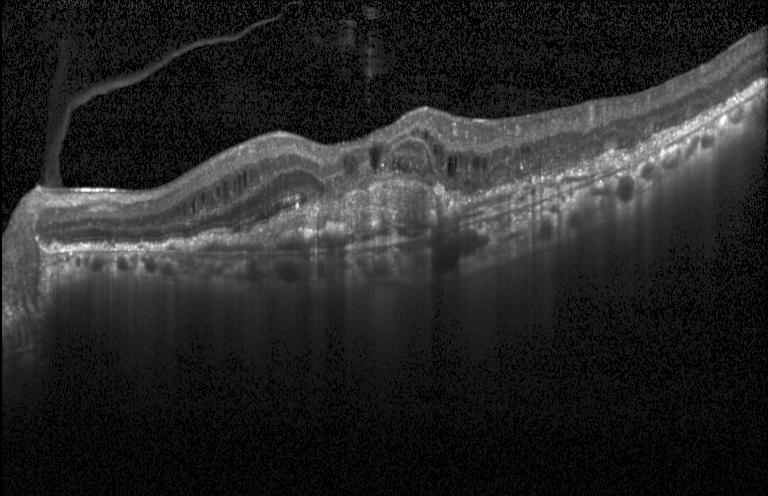
Spectral-domain optical coherence tomography · retinal OCT cross-section. Assessment: choroidal neovascularization (CNV).